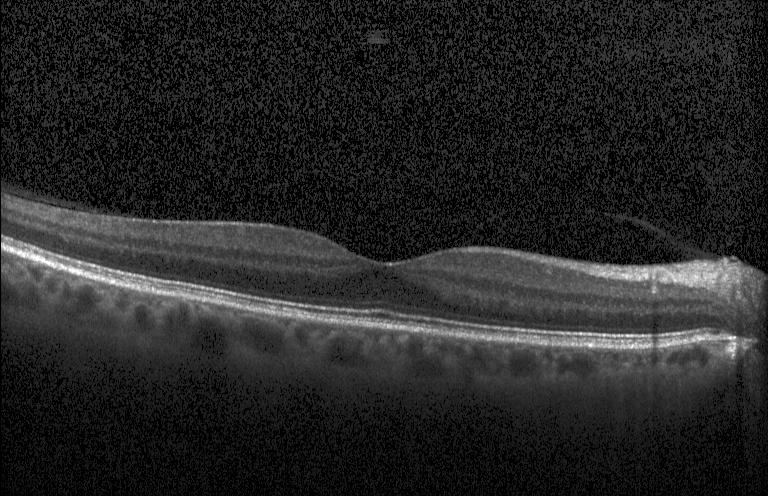 OCT B-scan.
Assessment: no choroidal neovascularization, diabetic macular edema, or drusen.